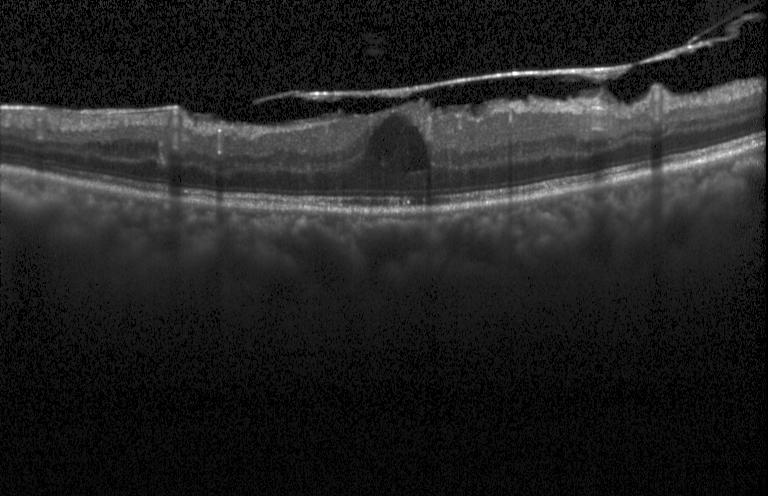
Dx: diabetic macular edema.